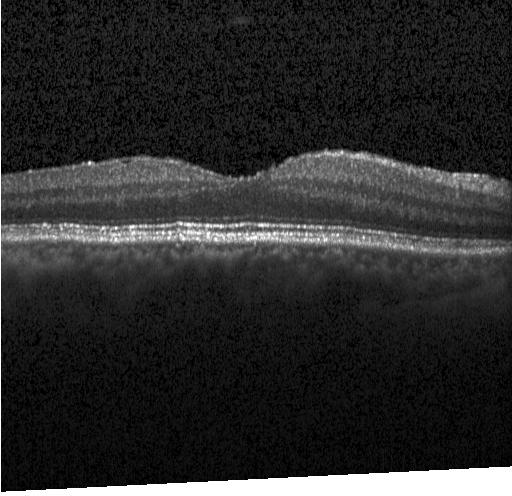
OCT line scan — Diagnosis: neither choroidal neovascularization, diabetic macular edema, nor drusen.